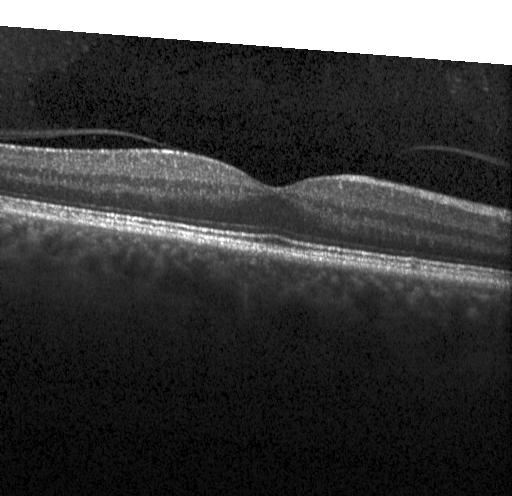 Instrument: Heidelberg Spectralis, optical coherence tomography scan, fovea-centered.
Impression: no choroidal neovascularization, no diabetic macular edema, and no drusen.